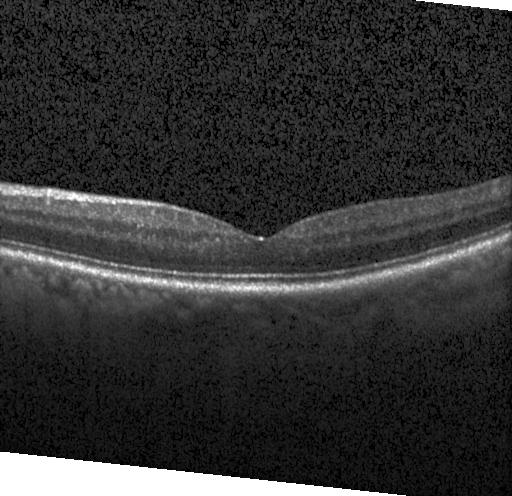
OCT line scan · through the macula — Dx: neither CNV, DME, nor drusen.